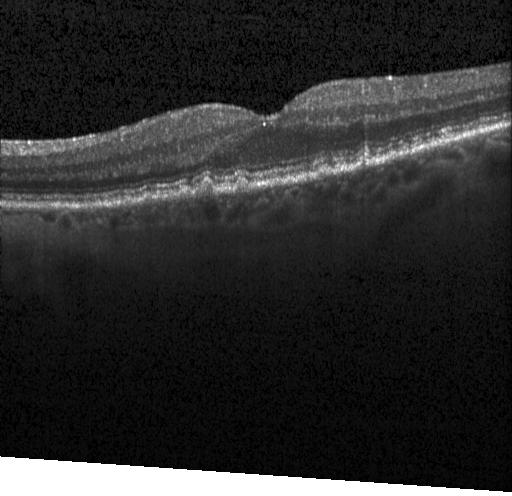

OCT scan showing multiple drusen.